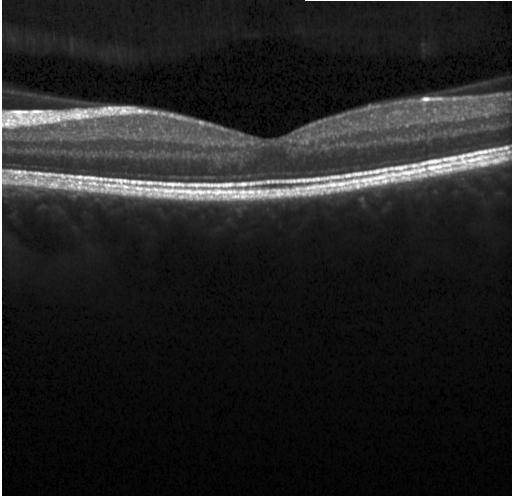
SD-OCT; optical coherence tomography B-scan; horizontal scan through the fovea.
Impression: neither choroidal neovascularization, diabetic macular edema, nor drusen.